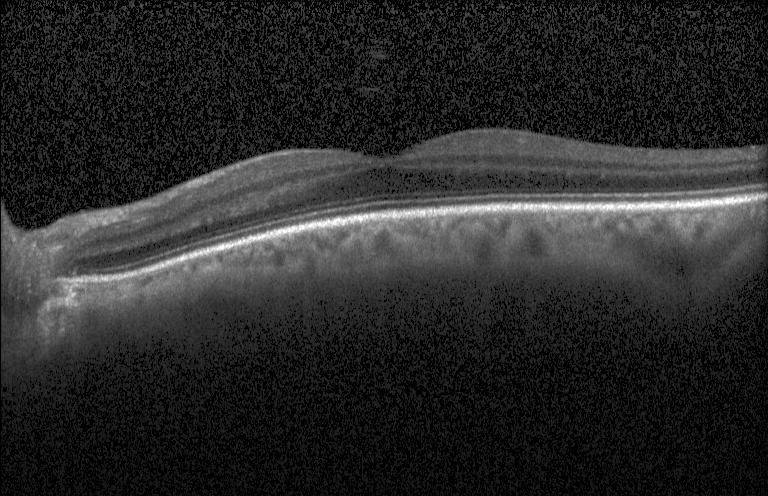

Assessment: no choroidal neovascularization, diabetic macular edema, or drusen.